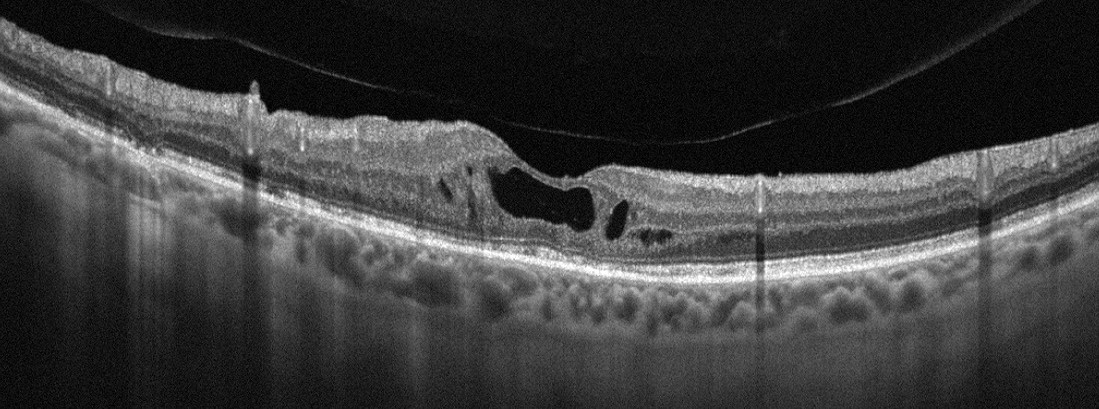 OCT finding: diabetic macular edema.